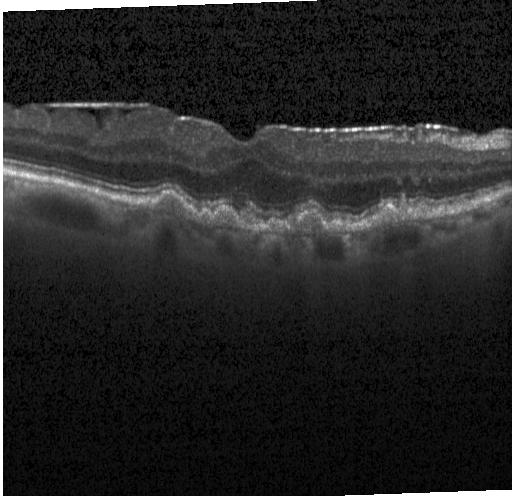
Optical coherence tomography scan.
Finding: drusen.